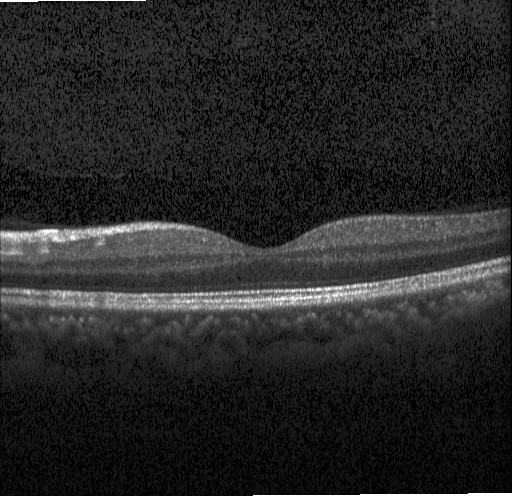

Spectral-domain OCT B-scan: no CNV, DME, or drusen.